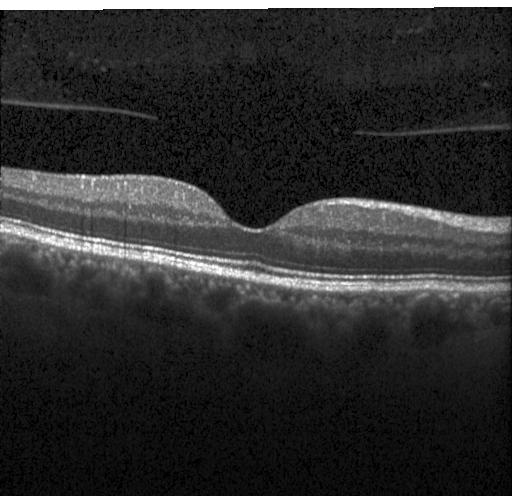

Heidelberg Spectralis, fovea-centered, OCT line scan.
Diagnosis: no CNV, no DME, and no drusen.